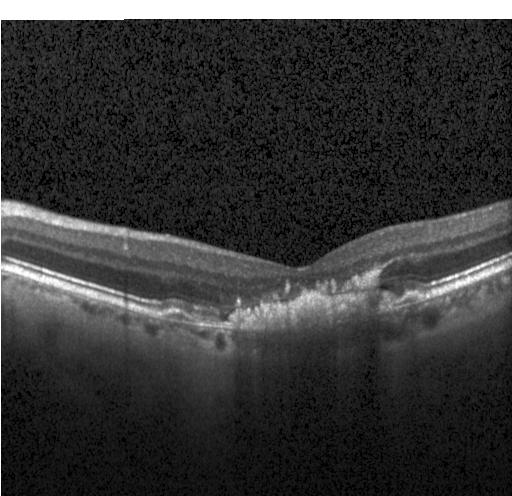

Spectral-domain OCT. Optical coherence tomography B-scan. Through the macula
Impression: choroidal neovascularization (CNV).